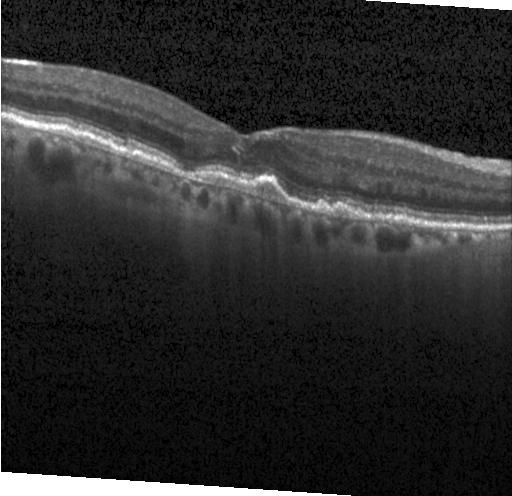 Diagnosis: choroidal neovascularization (CNV).